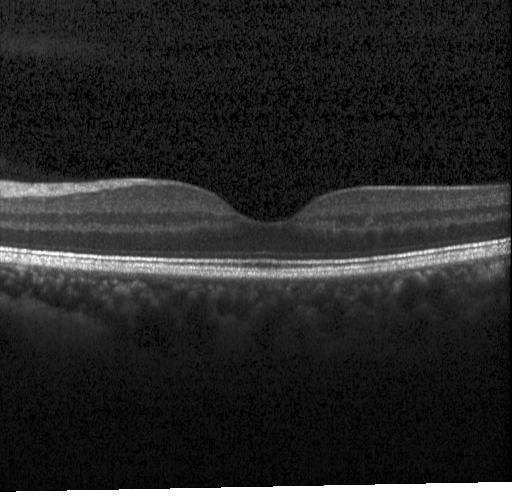 Retinal OCT B-scan · spectral-domain OCT
Finding: neither choroidal neovascularization, diabetic macular edema, nor drusen.